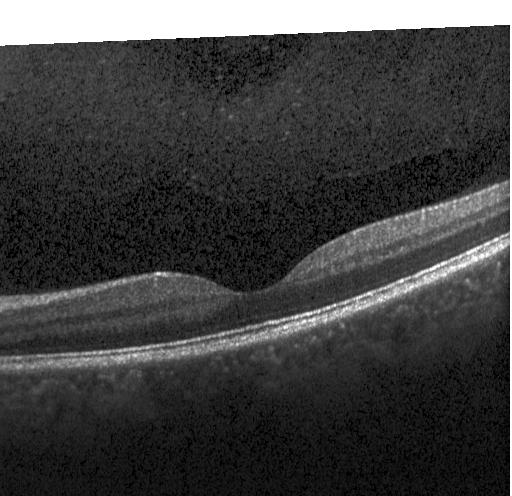 This B-scan demonstrates neither CNV, DME, nor drusen.